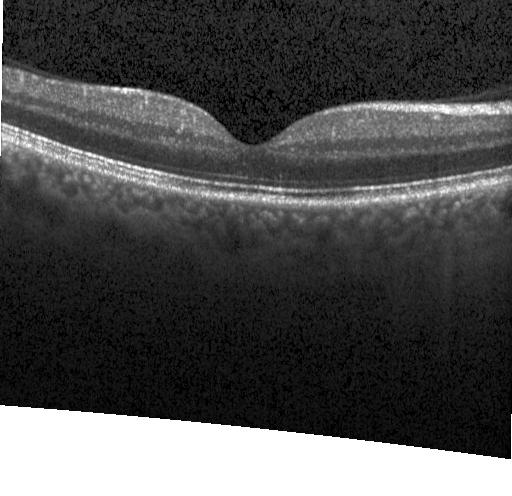

Macular OCT demonstrating neither CNV, DME, nor drusen.